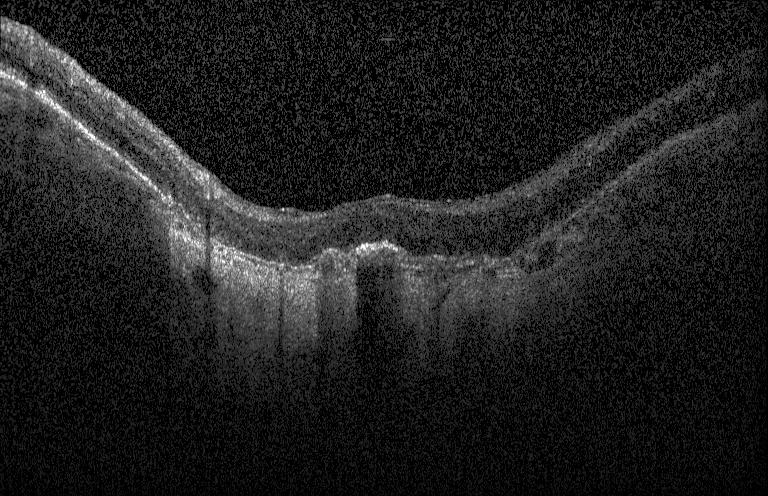
Macular OCT: choroidal neovascularization (CNV).